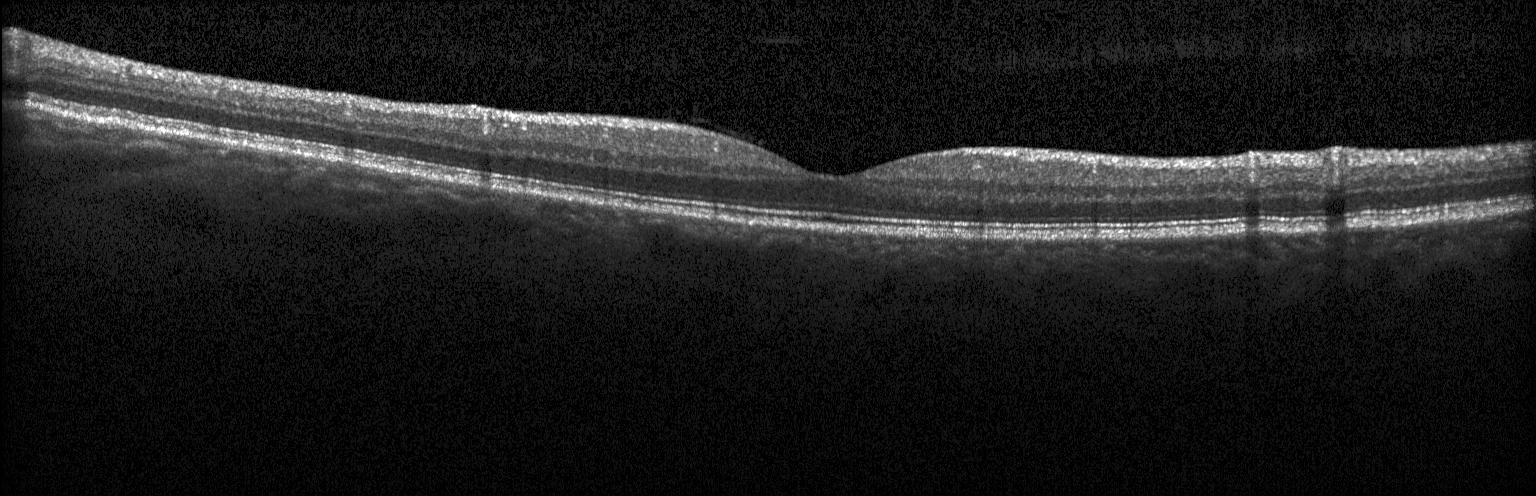
Retinal OCT cross-section.
Finding: no choroidal neovascularization, no diabetic macular edema, and no drusen.